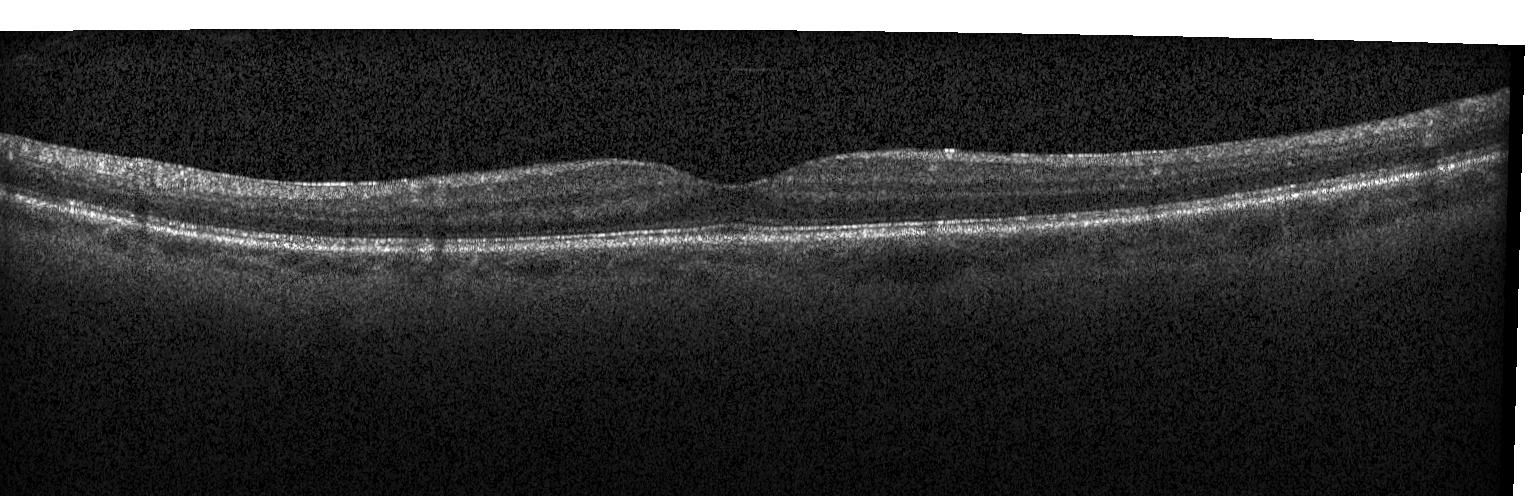
Centered on the fovea. Optical coherence tomography scan. Heidelberg Spectralis OCT system. SD-OCT
Diagnosis: no CNV, no DME, and no drusen.